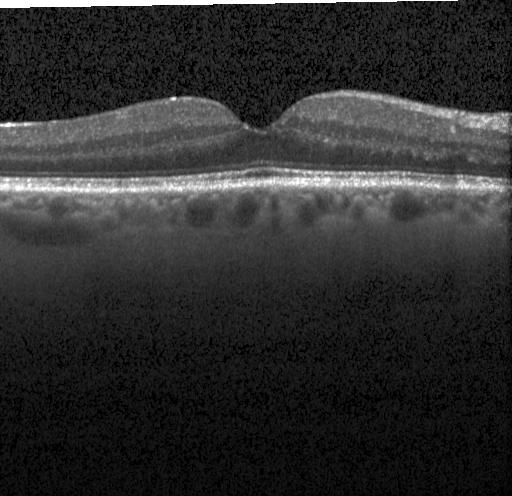

Horizontal scan through the fovea. OCT line scan.
Diagnosis: no choroidal neovascularization, no diabetic macular edema, and no drusen.